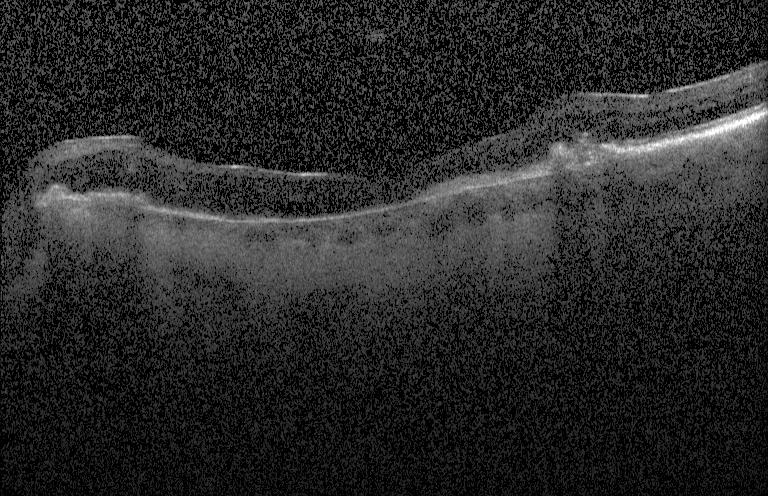 OCT B-scan, Heidelberg Spectralis OCT system
Assessment: a choroidal neovascular membrane.